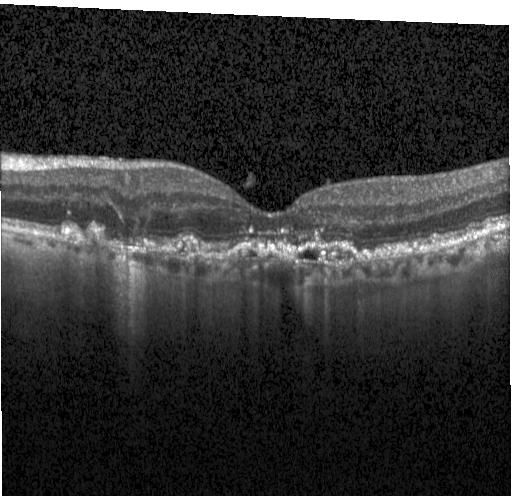
Macular OCT demonstrating choroidal neovascularization (CNV).